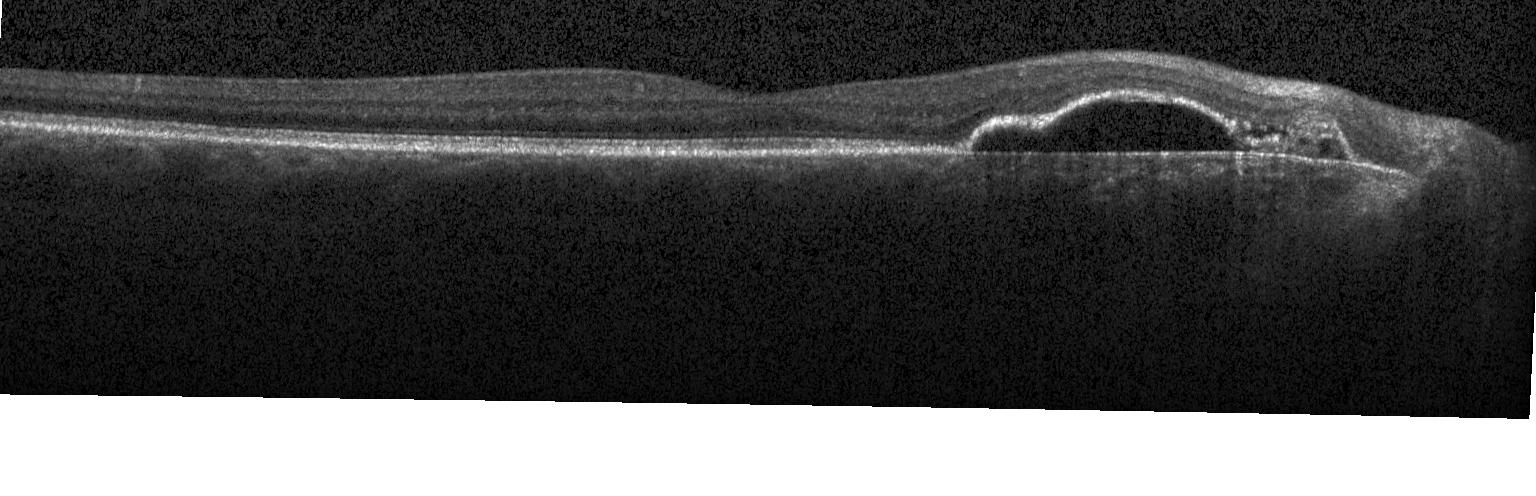
Instrument: Heidelberg Spectralis, horizontal scan through the fovea, spectral-domain optical coherence tomography, retinal OCT B-scan. The scan shows a choroidal neovascular membrane.